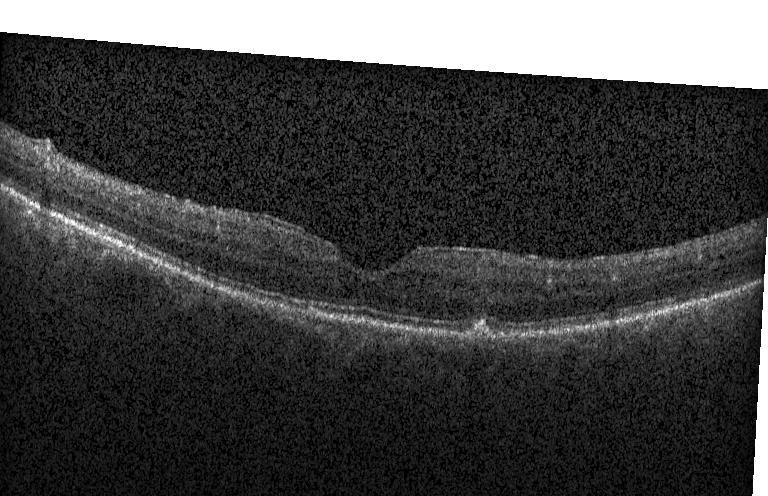 Finding: multiple drusen.